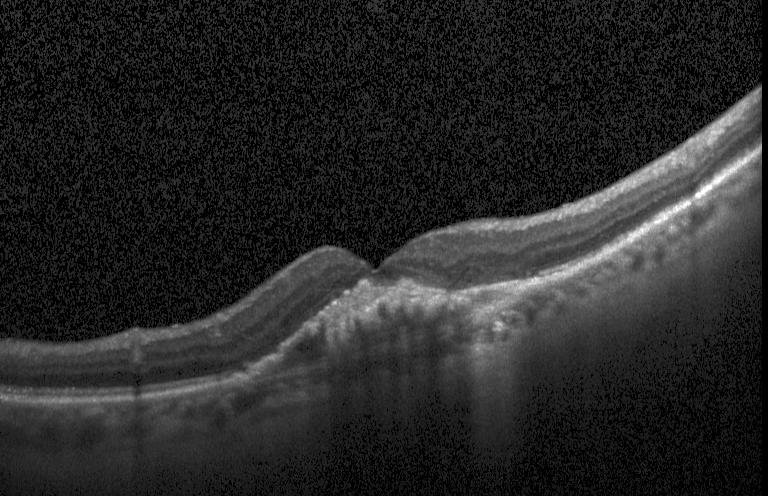

Fovea-centered; optical coherence tomography scan.
Diagnosis: choroidal neovascularization (CNV).